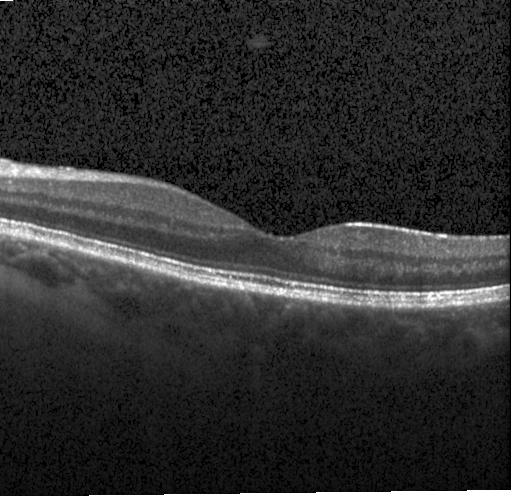 Optical coherence tomography scan; through the macula; spectral-domain OCT; Heidelberg Spectralis. Dx: no choroidal neovascularization, no diabetic macular edema, and no drusen.